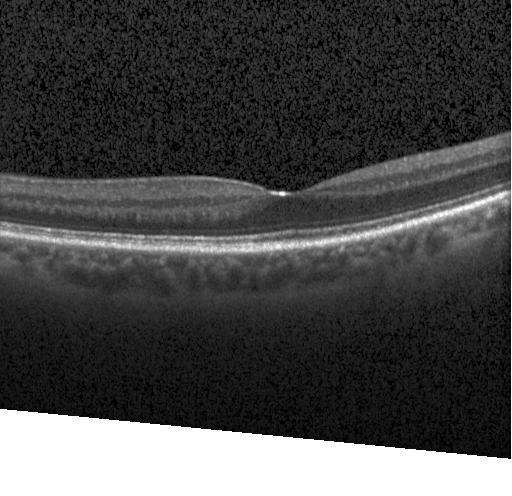

OCT line scan — OCT finding: neither choroidal neovascularization, diabetic macular edema, nor drusen.